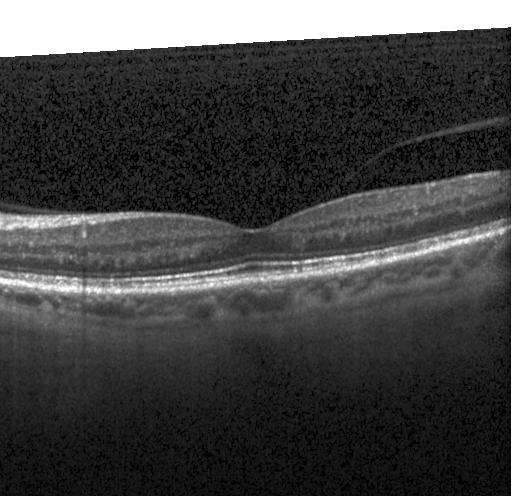 Optical coherence tomography scan. Diagnosis: neither choroidal neovascularization, diabetic macular edema, nor drusen.